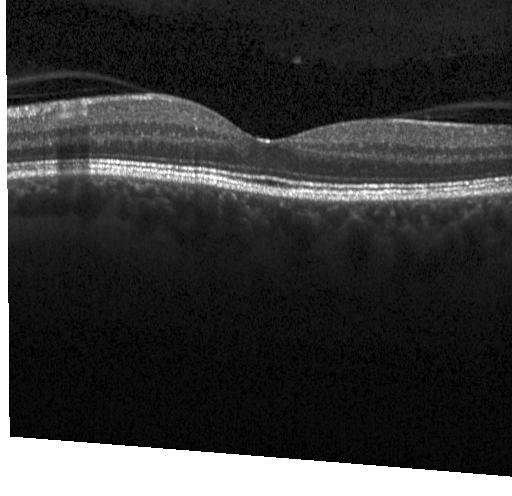

SD-OCT, optical coherence tomography B-scan.
Macular OCT: no choroidal neovascularization, no diabetic macular edema, and no drusen.